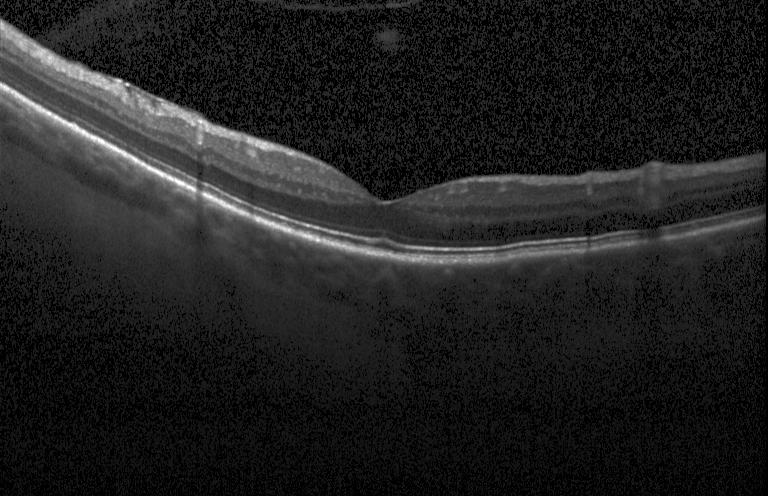 Optical coherence tomography B-scan. Instrument: Heidelberg Spectralis. Through the macula.
Finding: no CNV, no DME, and no drusen.